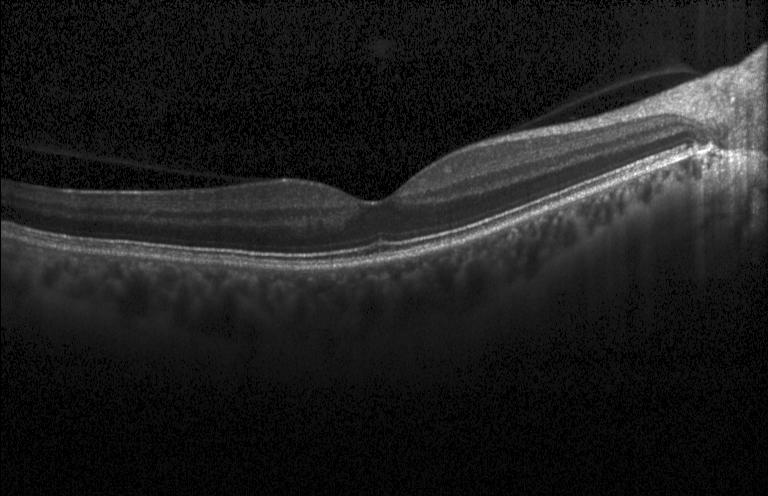
SD-OCT · instrument: Heidelberg Spectralis · macular scan · retinal OCT B-scan. Finding: neither choroidal neovascularization, diabetic macular edema, nor drusen.